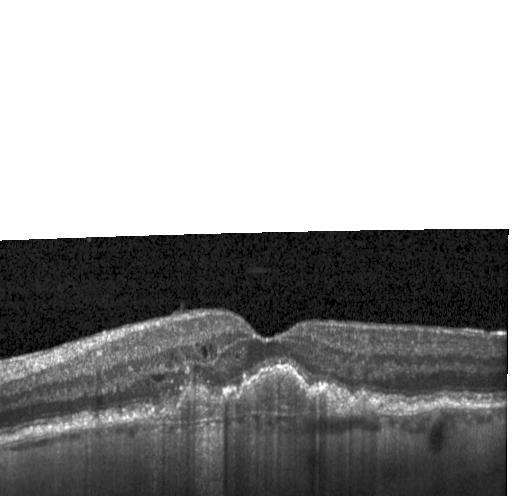
OCT scan showing a choroidal neovascular membrane.